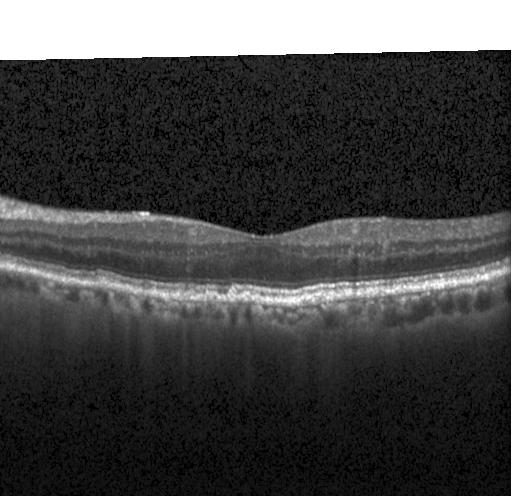

Heidelberg Spectralis. Spectral-domain optical coherence tomography. OCT B-scan. Fovea-centered. Dx: sub-RPE drusenoid deposits.